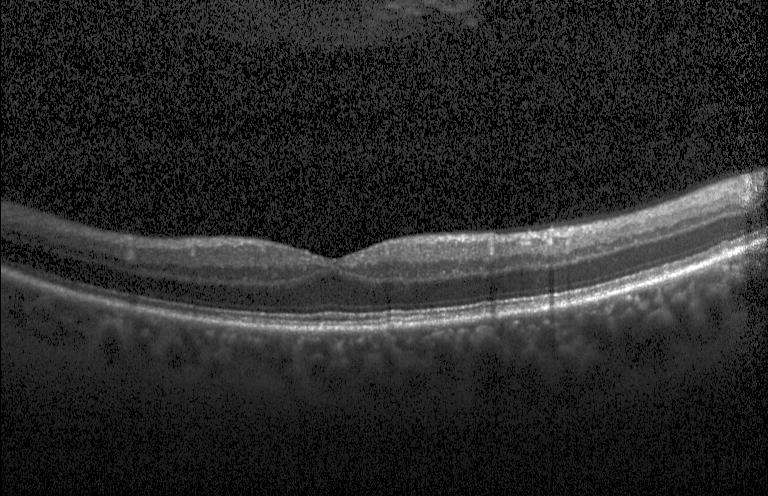 Diagnosis: no evidence of CNV, DME, or drusen.